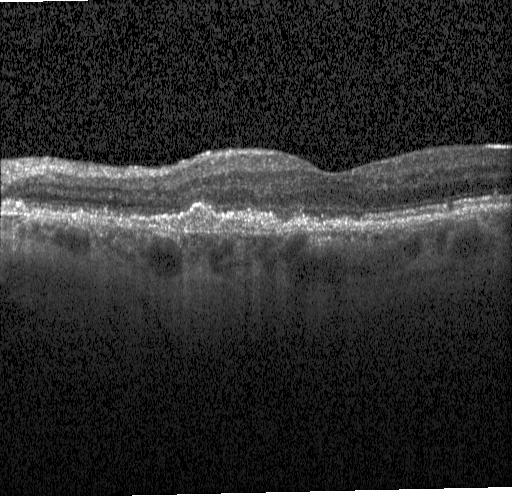 This B-scan demonstrates a choroidal neovascular membrane.